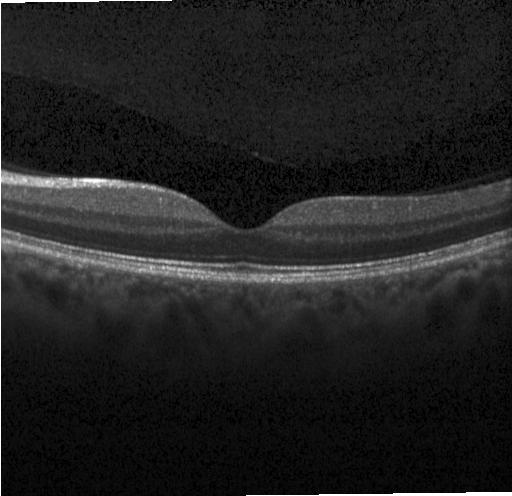
Macular OCT demonstrating no choroidal neovascularization, no diabetic macular edema, and no drusen.